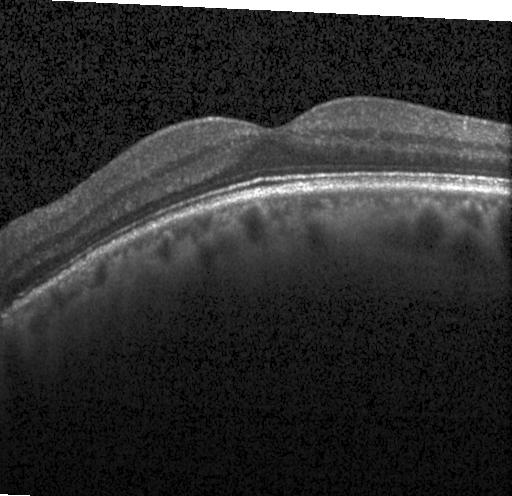

Optical coherence tomography B-scan. Through the macula
Finding: no choroidal neovascularization, no diabetic macular edema, and no drusen.